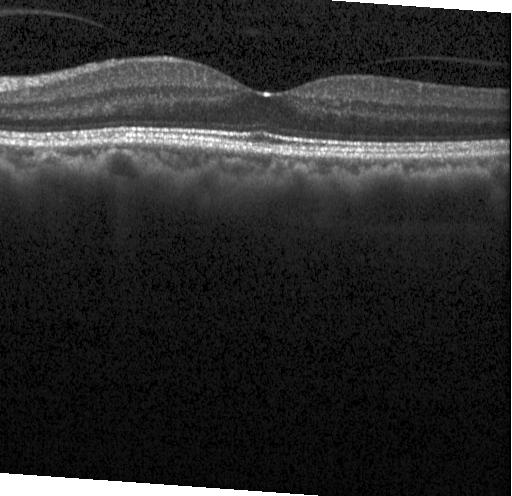 OCT B-scan — The scan shows no choroidal neovascularization, diabetic macular edema, or drusen.